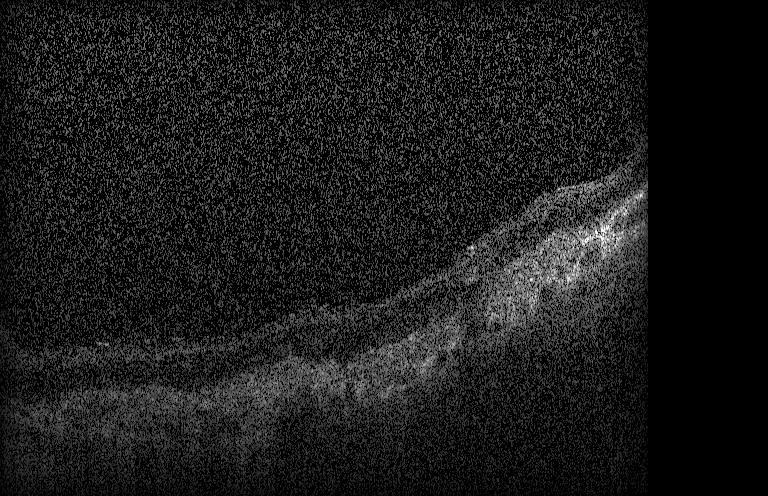
OCT finding: choroidal neovascularization.